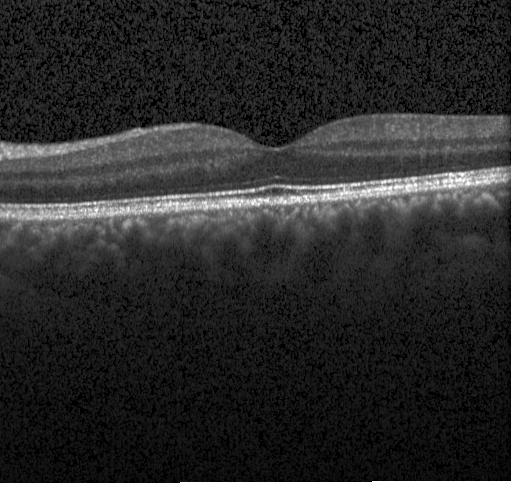

Centered on the fovea · retinal OCT cross-section
The scan shows no evidence of choroidal neovascularization, diabetic macular edema, or drusen.